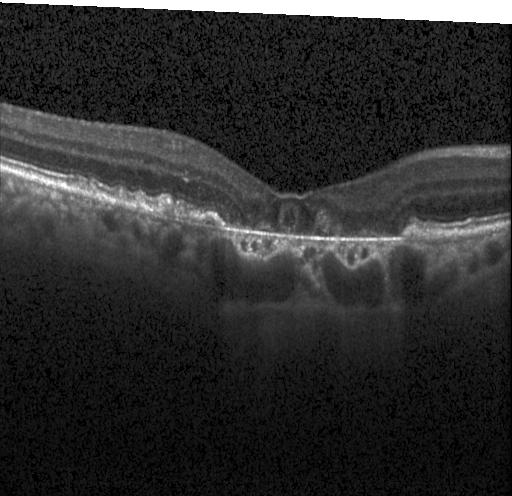 Optical coherence tomography scan, SD-OCT
This B-scan demonstrates CNV.